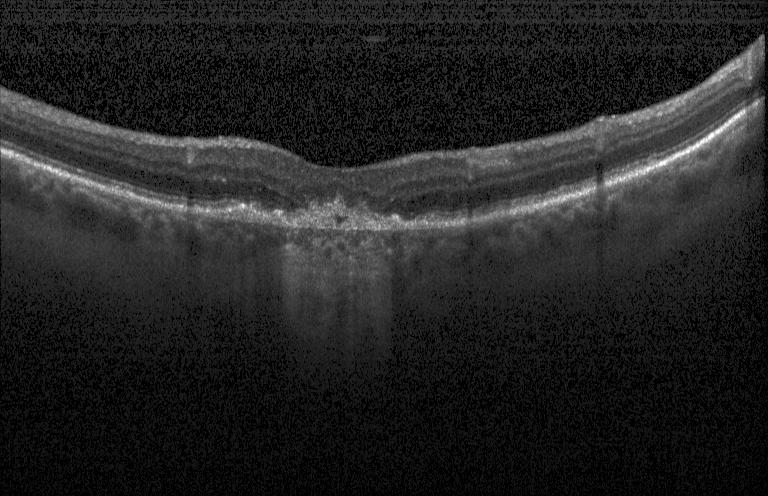 Optical coherence tomography scan — Assessment: choroidal neovascularization (CNV).